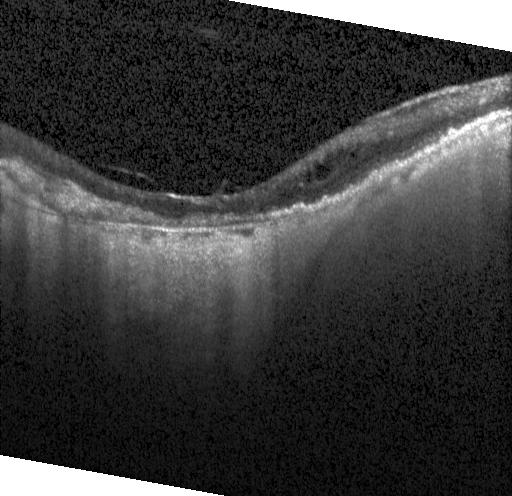 The scan shows choroidal neovascularization (CNV).